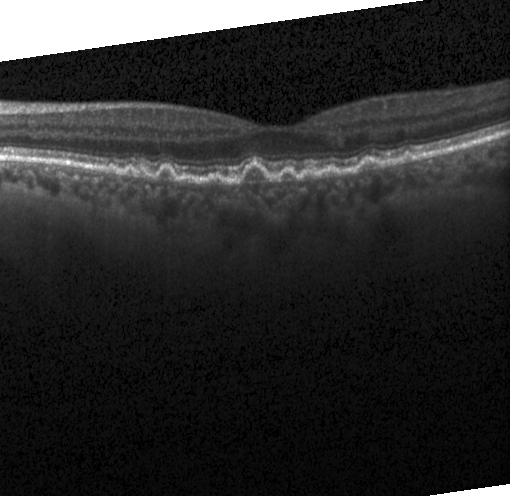 Retinal OCT cross-section showing drusen.